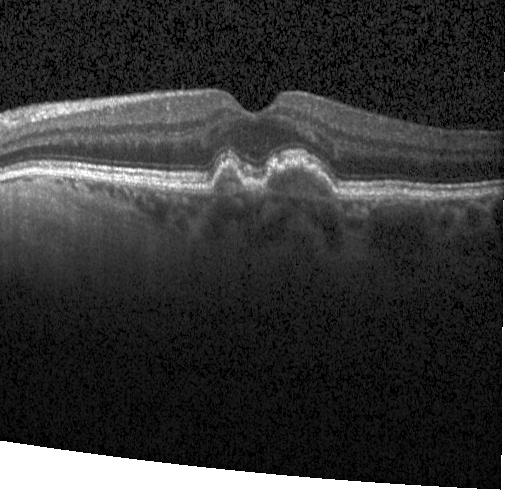

Spectral-domain OCT B-scan: choroidal neovascularization.